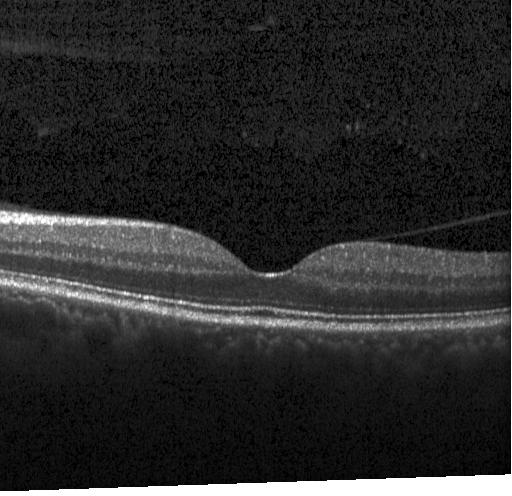
Macular OCT: no CNV, no DME, and no drusen.